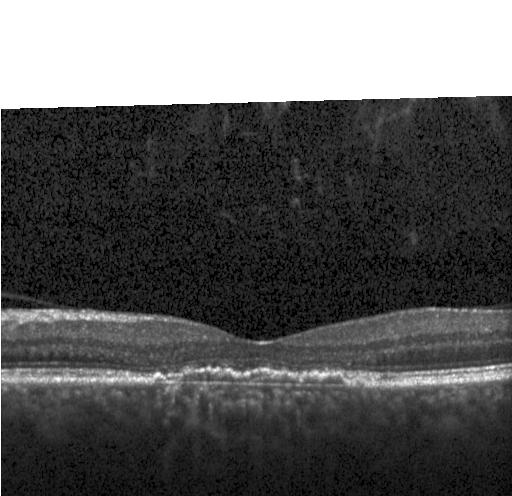
Retinal OCT B-scan; horizontal scan through the fovea; SD-OCT — Diagnosis: choroidal neovascularization.